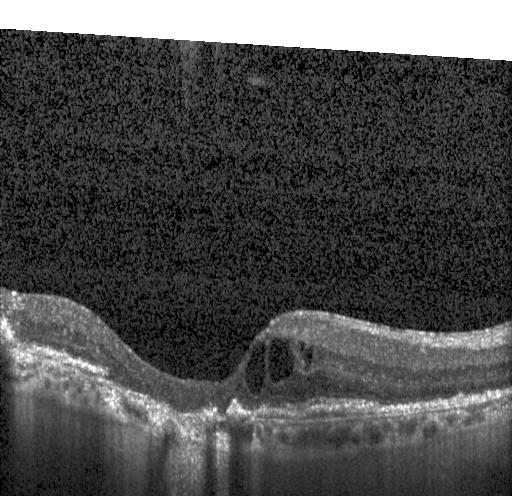 OCT line scan.
Assessment: CNV.